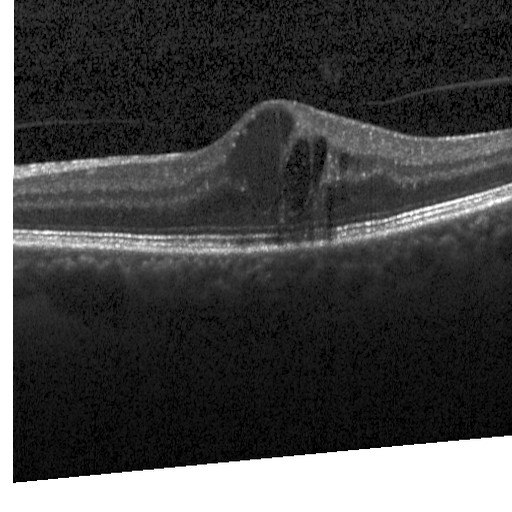

SD-OCT · Heidelberg Spectralis · OCT B-scan
Dx: DME.